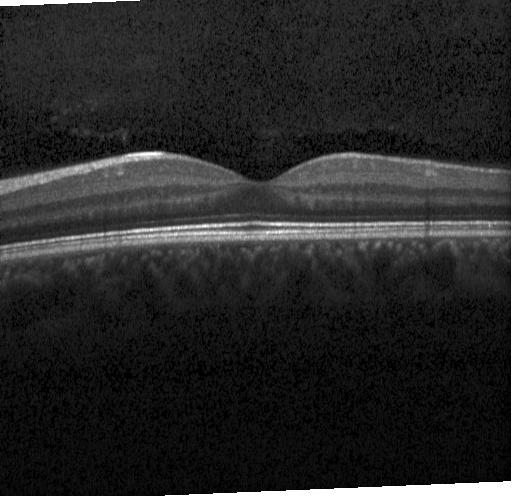
Dx: no evidence of choroidal neovascularization, diabetic macular edema, or drusen.